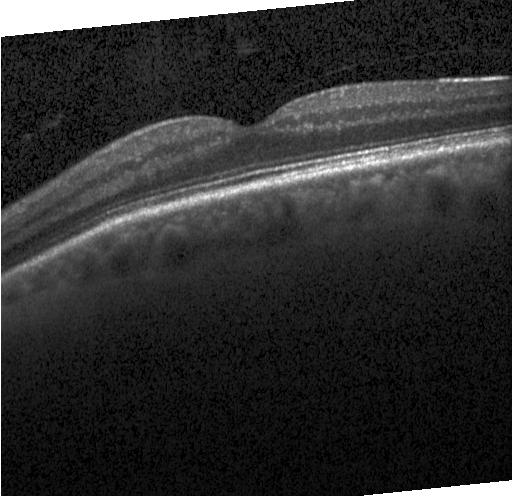

This B-scan demonstrates neither choroidal neovascularization, diabetic macular edema, nor drusen.